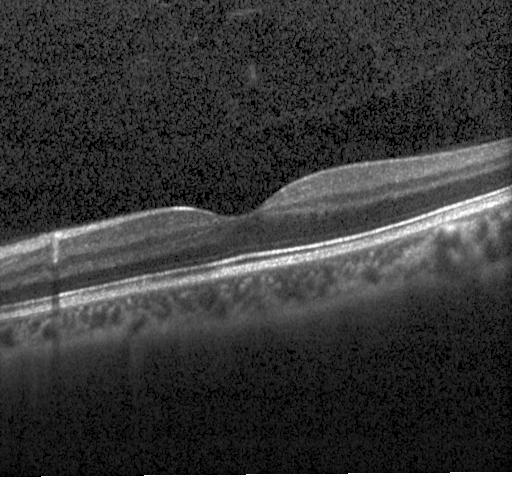

Acquired on a Heidelberg Spectralis, retinal OCT cross-section — Macular OCT: no evidence of choroidal neovascularization, diabetic macular edema, or drusen.